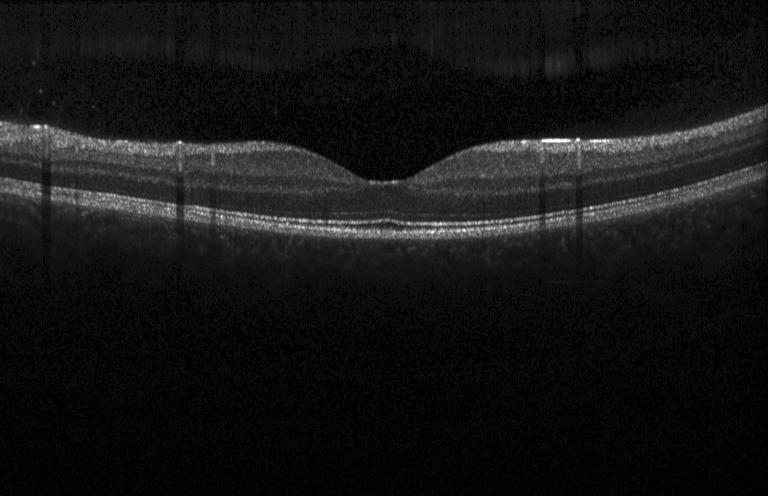 Spectral-domain OCT; optical coherence tomography scan. Macular OCT: no evidence of choroidal neovascularization, diabetic macular edema, or drusen.